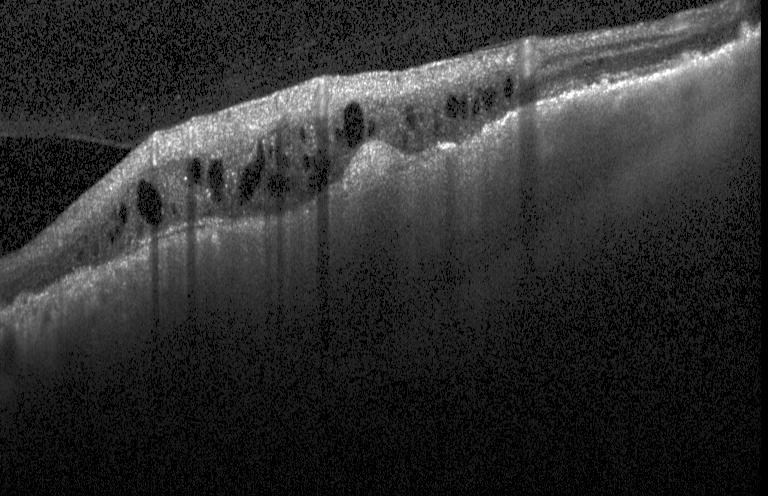 Centered on the fovea. Optical coherence tomography scan
Diagnosis: CNV.